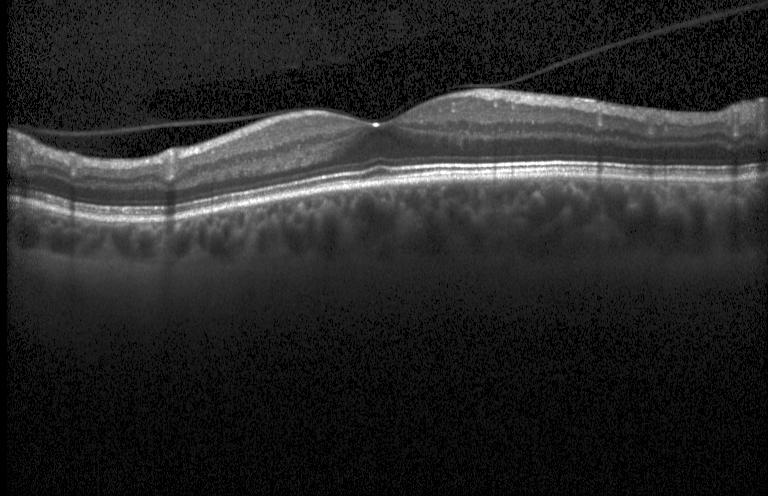
OCT B-scan showing neither choroidal neovascularization, diabetic macular edema, nor drusen.